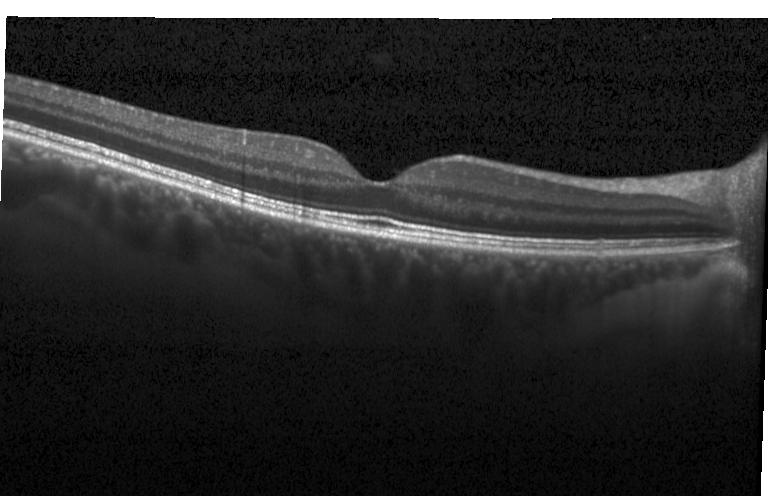

Macular scan. Retinal OCT cross-section. Spectral-domain optical coherence tomography. Heidelberg Spectralis OCT system. Neither CNV, DME, nor drusen.